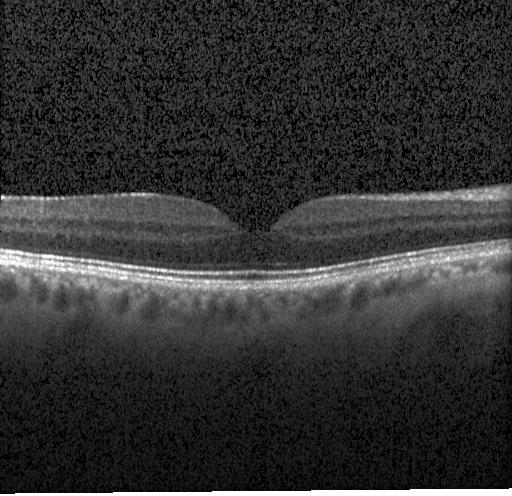 Spectral-domain OCT B-scan: no evidence of choroidal neovascularization, diabetic macular edema, or drusen.